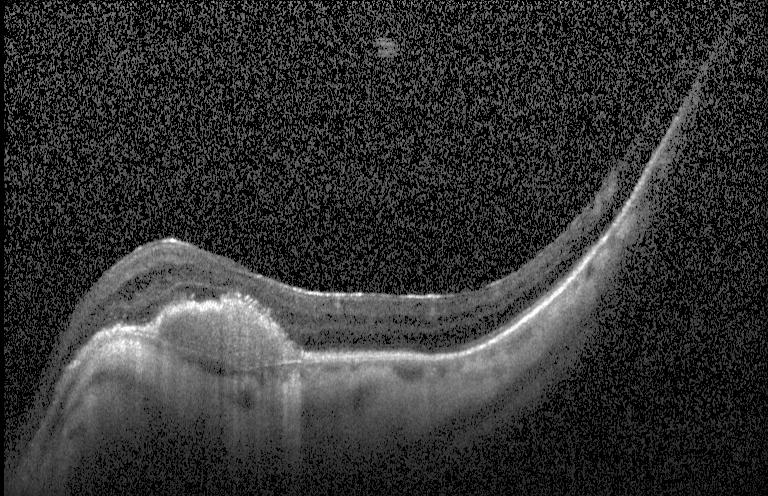
Retinal OCT B-scan
OCT finding: choroidal neovascularization (CNV).